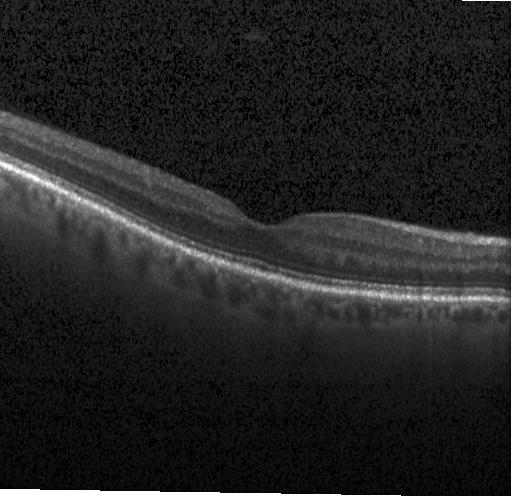
Diagnosis: no CNV, no DME, and no drusen.